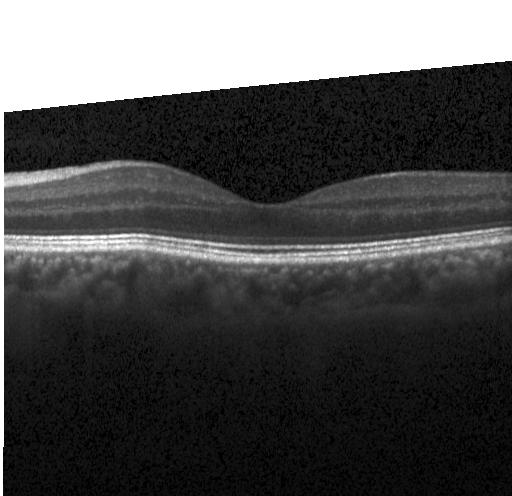

SD-OCT, optical coherence tomography scan, through the macula, Heidelberg Spectralis.
Assessment: no CNV, DME, or drusen.